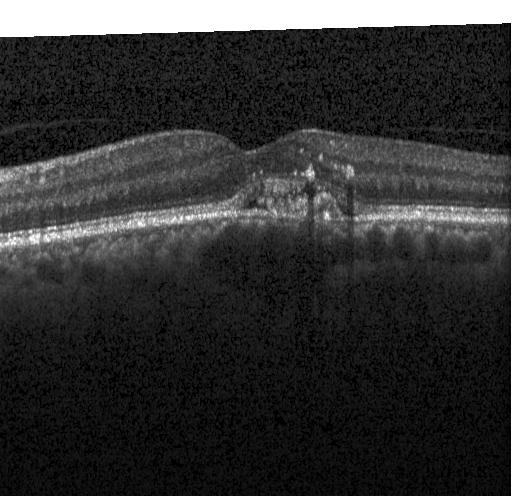 OCT B-scan showing a choroidal neovascular membrane.